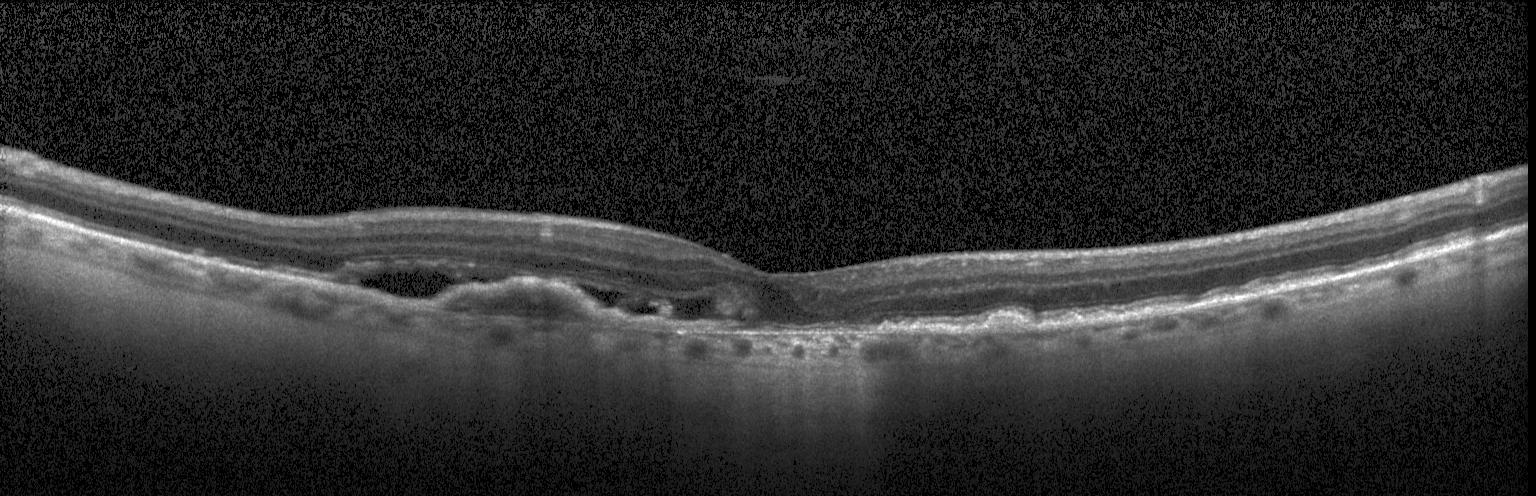 Optical coherence tomography B-scan.
Choroidal neovascularization.